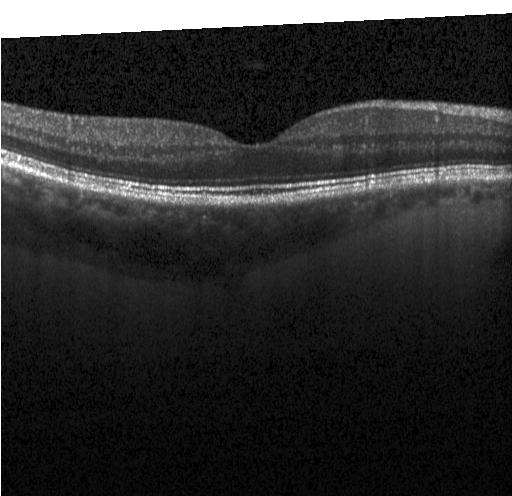

OCT B-scan showing neither CNV, DME, nor drusen.